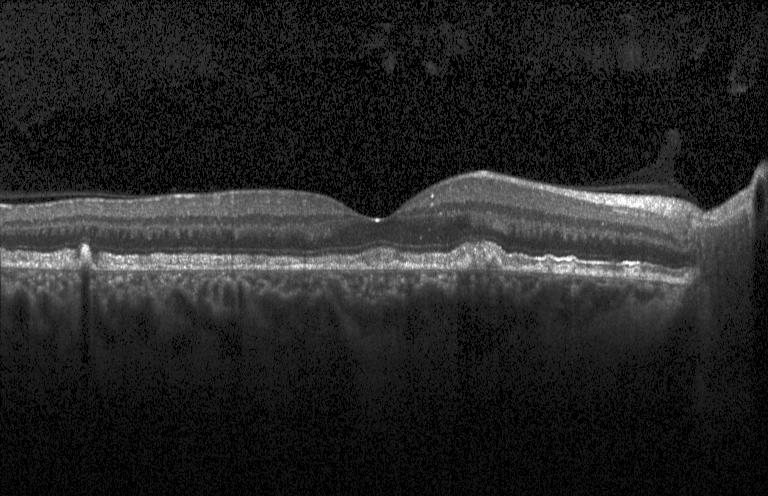
Diagnosis: drusen.